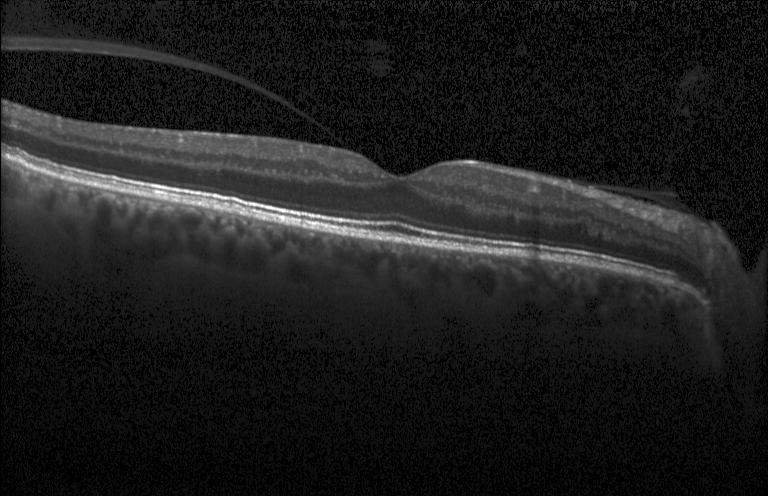
Retinal OCT cross-section, SD-OCT.
OCT finding: no choroidal neovascularization, diabetic macular edema, or drusen.